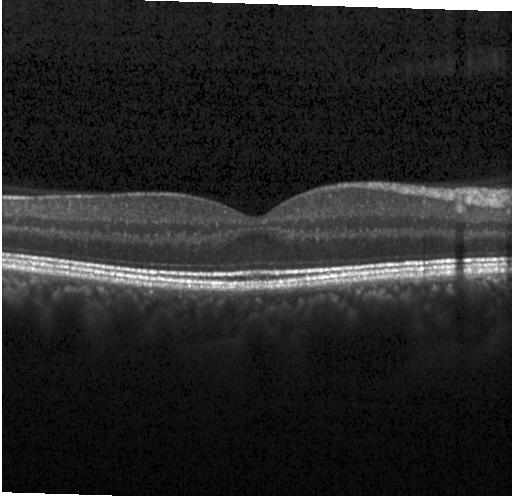
OCT line scan — Impression: no choroidal neovascularization, no diabetic macular edema, and no drusen.